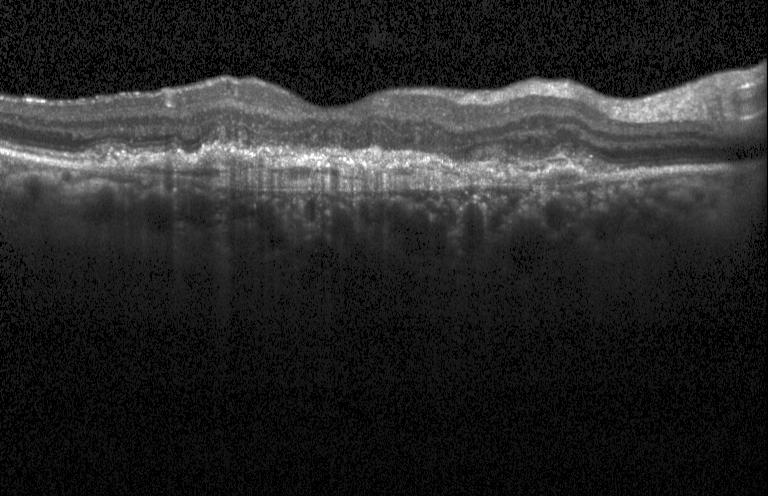
Retinal OCT cross-section, fovea-centered. This B-scan demonstrates choroidal neovascularization.